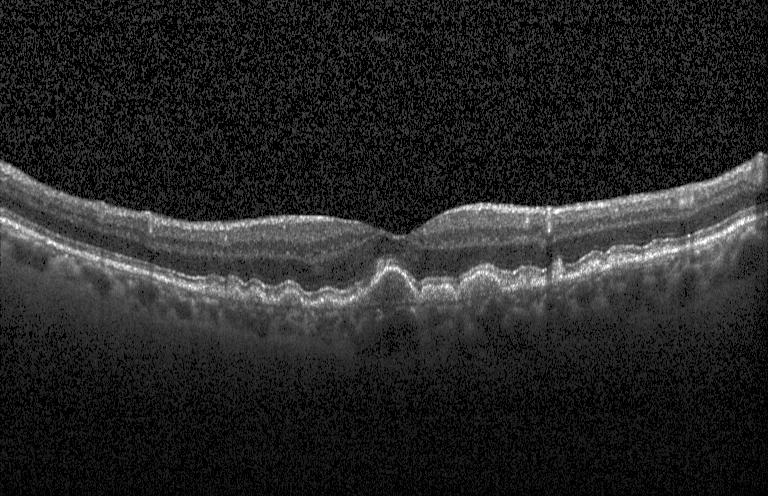
Centered on the fovea; optical coherence tomography B-scan; spectral-domain optical coherence tomography — Impression: sub-RPE drusenoid deposits.